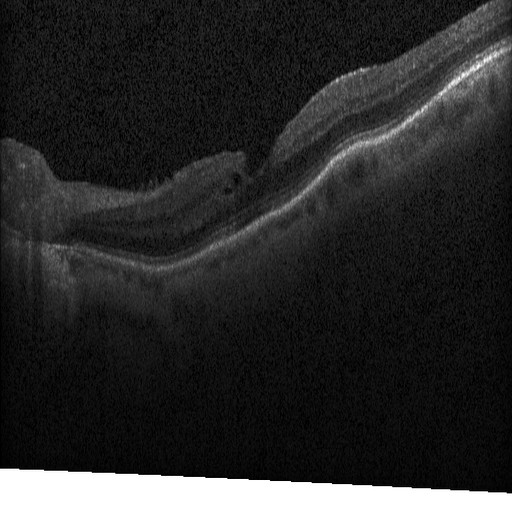
Retinal OCT cross-section; macular scan; Heidelberg Spectralis OCT system — This B-scan demonstrates diabetic macular edema.